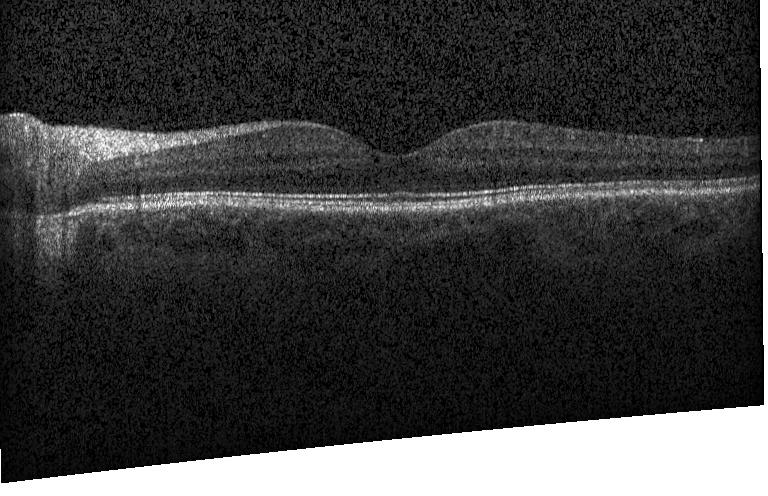

Retinal OCT cross-section · spectral-domain OCT · Heidelberg Spectralis · fovea-centered
The scan shows neither choroidal neovascularization, diabetic macular edema, nor drusen.